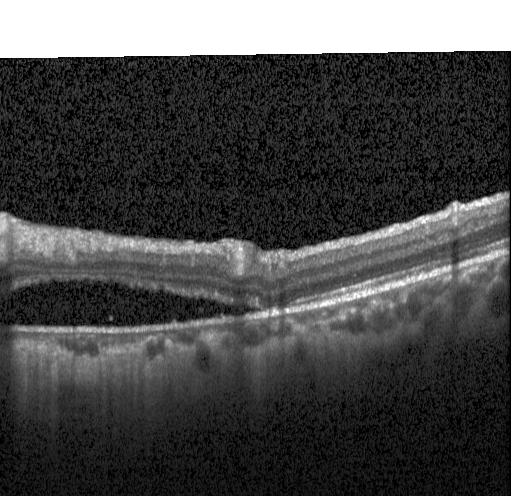

Dx: a choroidal neovascular membrane.